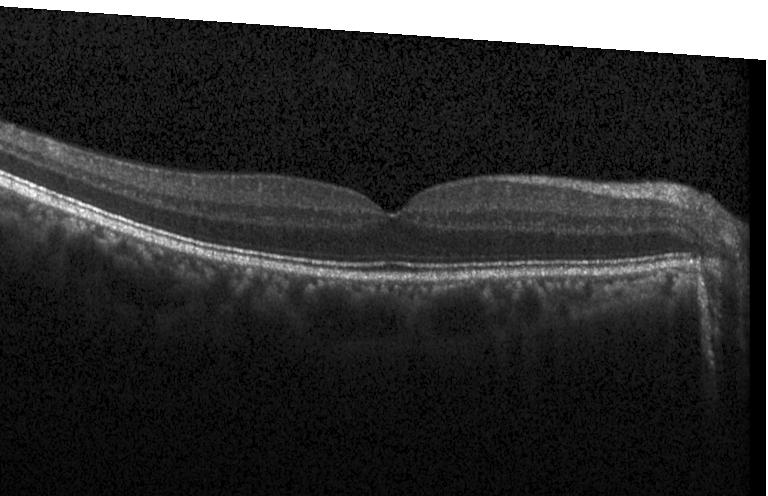

Macular OCT: no choroidal neovascularization, diabetic macular edema, or drusen.